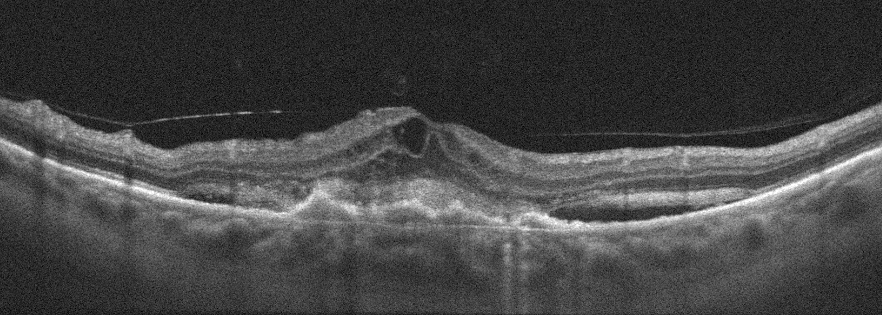 Retinal OCT B-scan · OS
Finding: age-related macular degeneration.